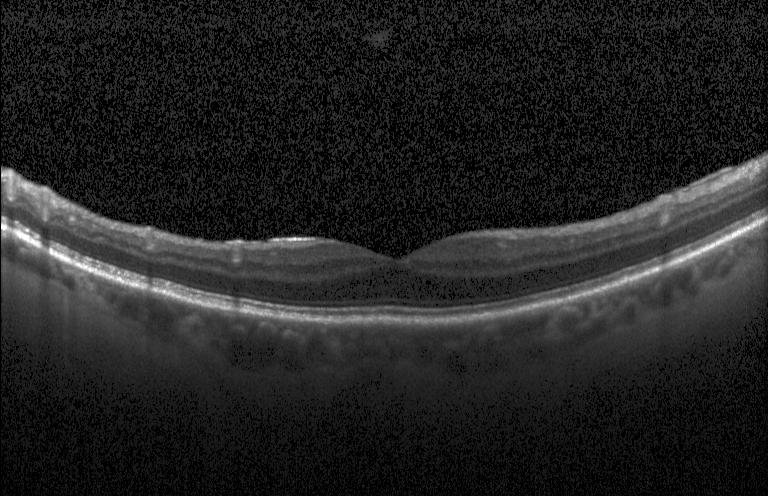
Finding: no choroidal neovascularization, no diabetic macular edema, and no drusen.